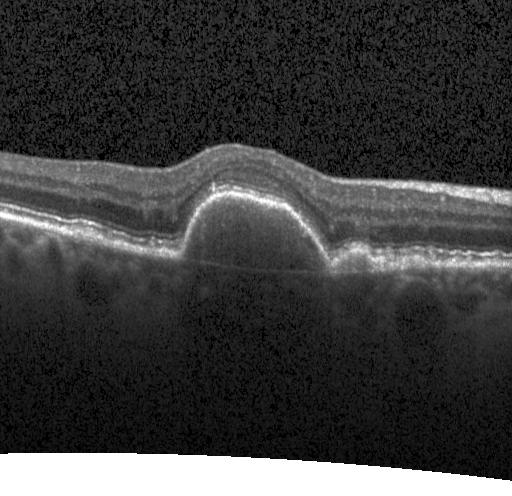 OCT B-scan — Diagnosis: a choroidal neovascular membrane.